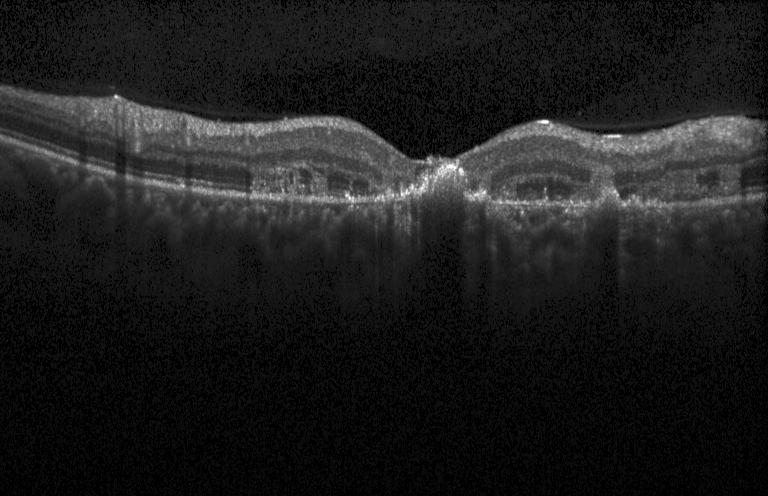
Spectral-domain OCT B-scan: a choroidal neovascular membrane.